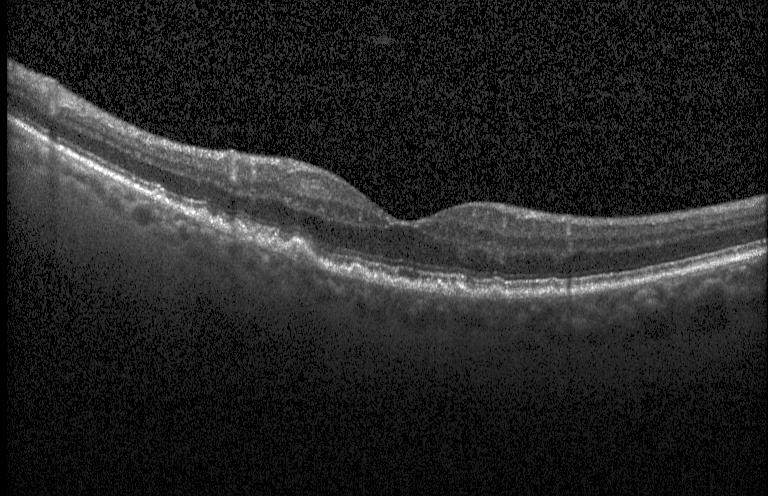 Diagnosis: sub-RPE drusenoid deposits.